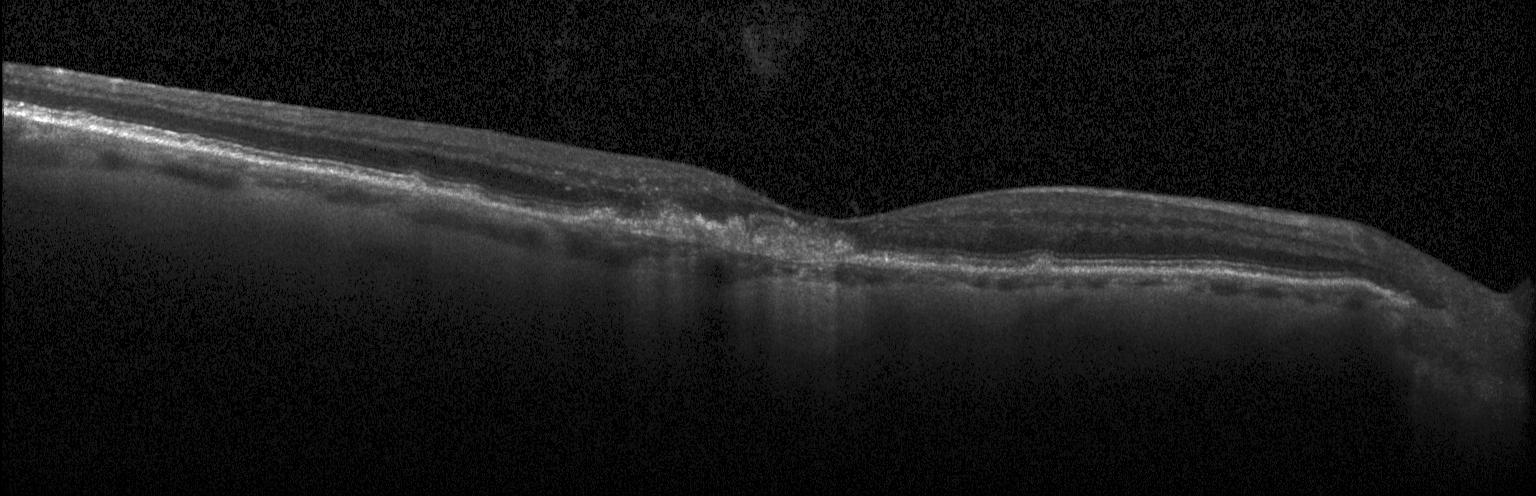
Finding: a choroidal neovascular membrane.